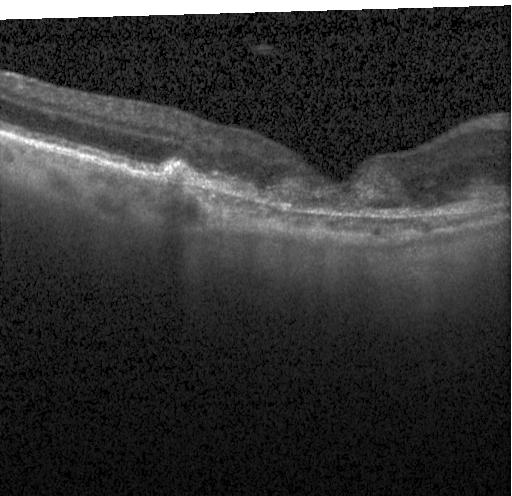

OCT finding: choroidal neovascularization.